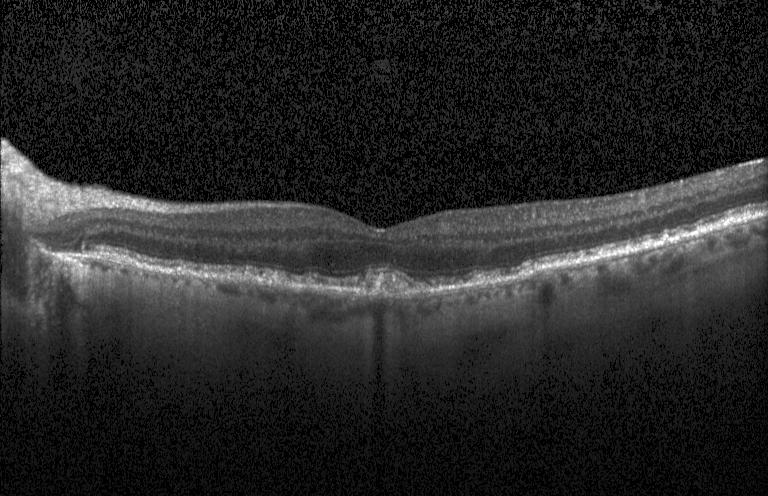 OCT finding: drusen.